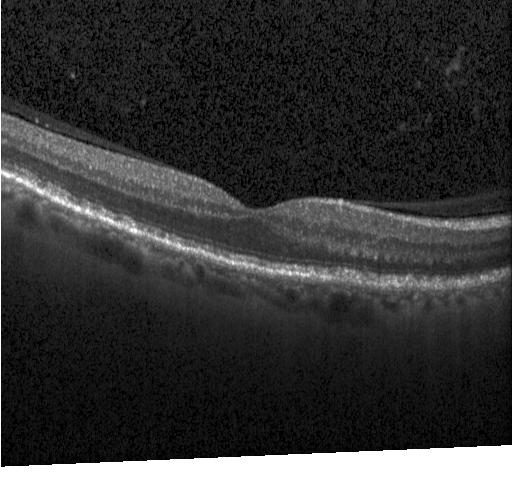 This B-scan demonstrates no choroidal neovascularization, diabetic macular edema, or drusen.